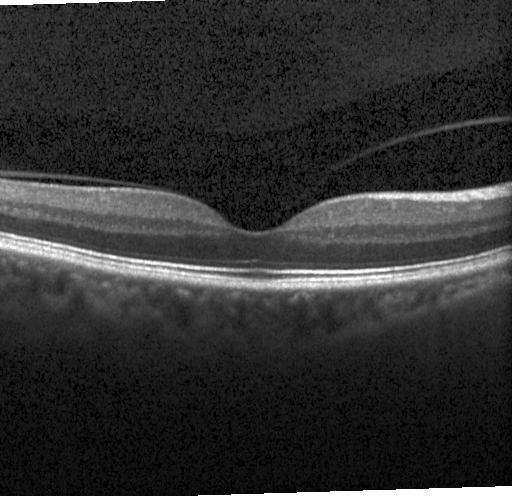 Optical coherence tomography B-scan. Instrument: Heidelberg Spectralis.
Dx: no evidence of choroidal neovascularization, diabetic macular edema, or drusen.